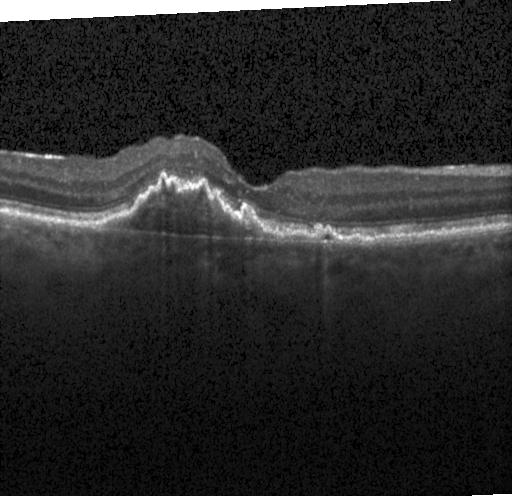 OCT finding: a choroidal neovascular membrane.